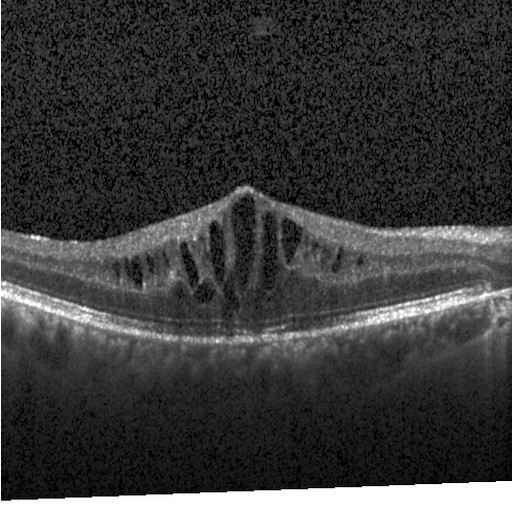 Heidelberg Spectralis; fovea-centered; spectral-domain optical coherence tomography; optical coherence tomography B-scan.
Finding: DME.